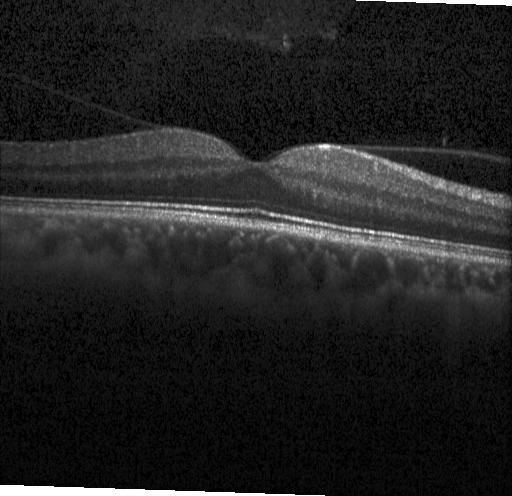 Retinal OCT B-scan; acquired on a Heidelberg Spectralis; through the macula.
OCT finding: neither choroidal neovascularization, diabetic macular edema, nor drusen.